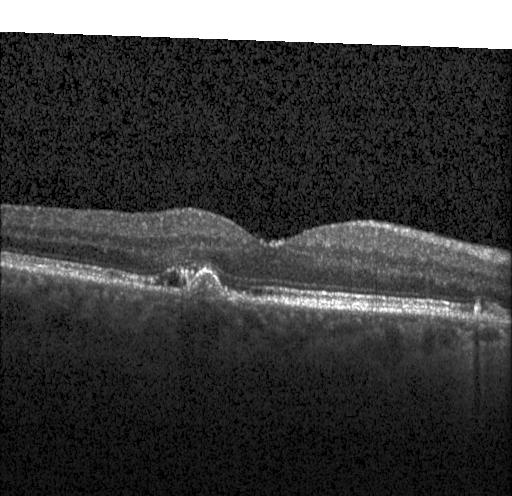
Impression: CNV.